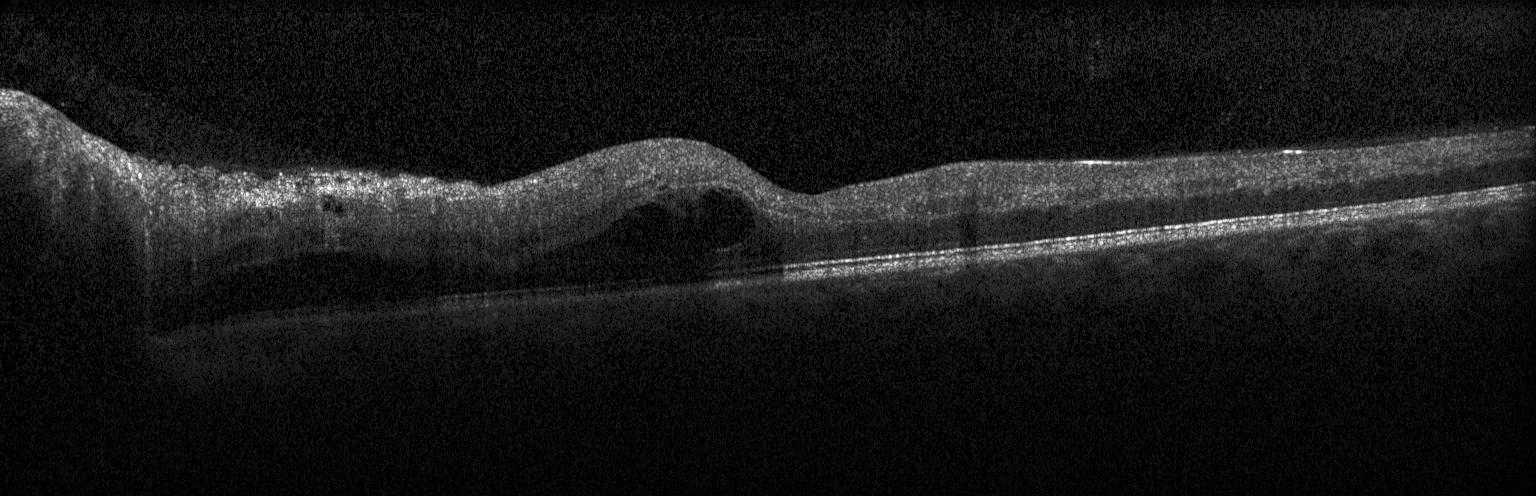 OCT line scan. Diabetic macular edema.